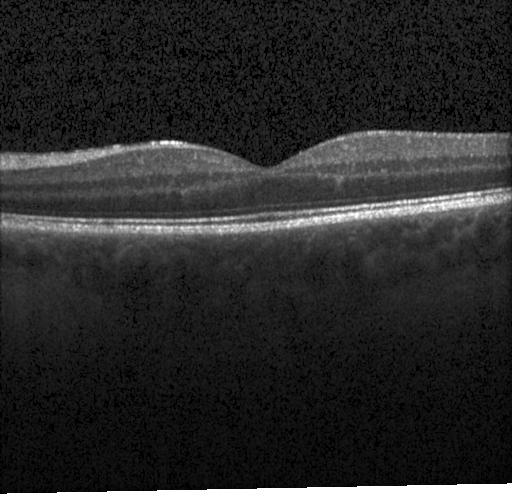

Heidelberg Spectralis OCT system. Optical coherence tomography scan. SD-OCT. No evidence of CNV, DME, or drusen.